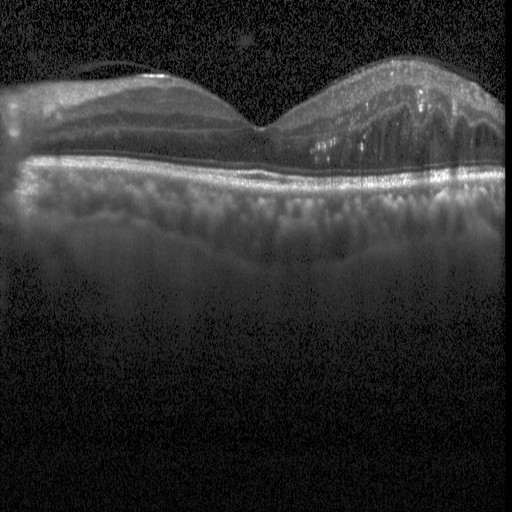

Finding: DME.